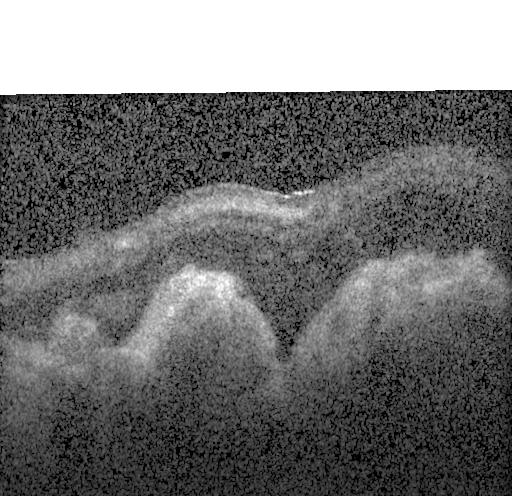 Spectral-domain OCT · retinal OCT B-scan · acquired on a Heidelberg Spectralis
Choroidal neovascularization (CNV).